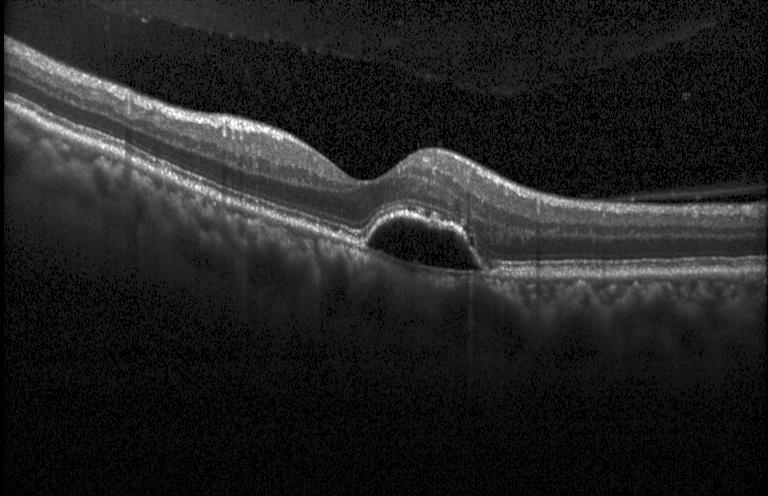 OCT B-scan, spectral-domain optical coherence tomography, acquired on a Heidelberg Spectralis
This B-scan demonstrates CNV.